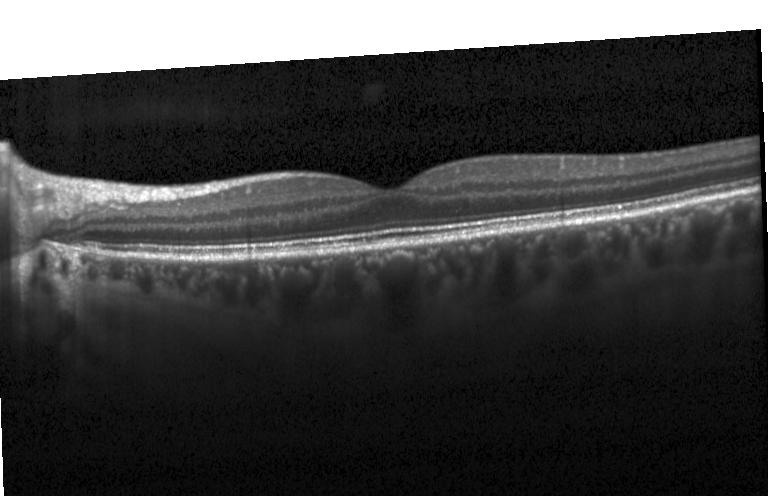
Diagnosis: neither choroidal neovascularization, diabetic macular edema, nor drusen.